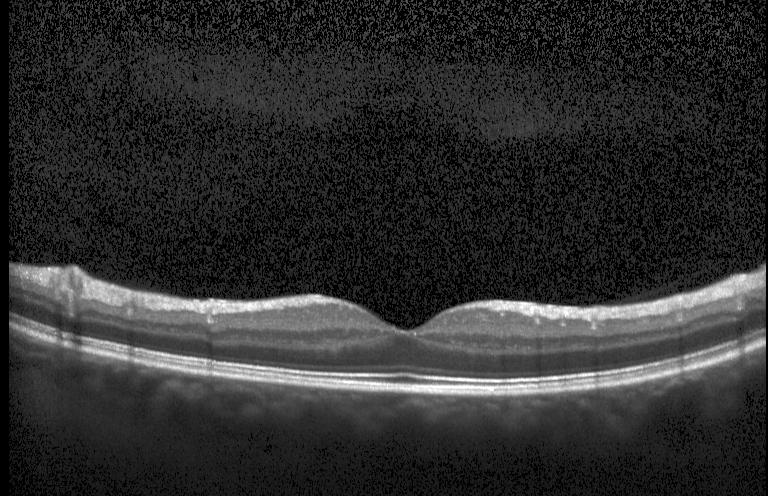 Heidelberg Spectralis. Optical coherence tomography scan. Spectral-domain optical coherence tomography — Diagnosis: no evidence of choroidal neovascularization, diabetic macular edema, or drusen.